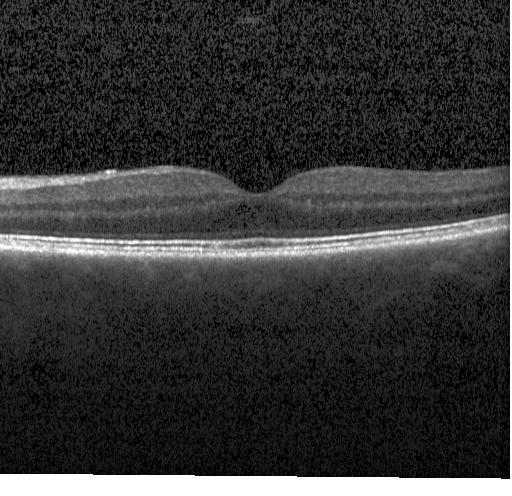

Centered on the fovea; OCT line scan.
Impression: no choroidal neovascularization, no diabetic macular edema, and no drusen.